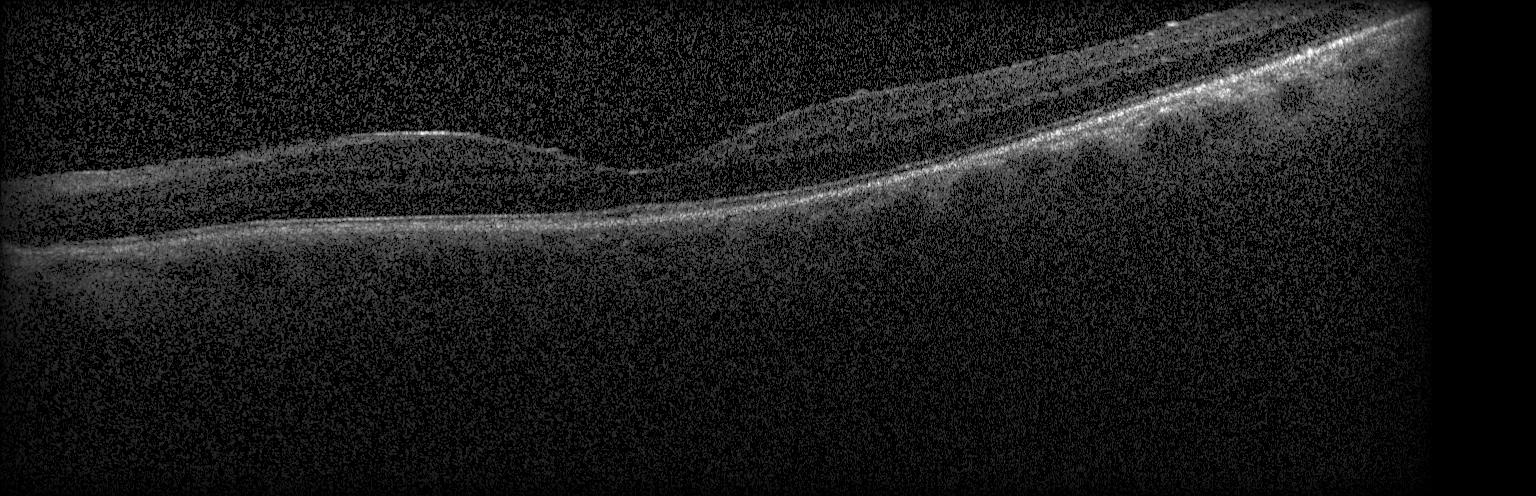

Spectral-domain OCT, macular scan, acquired on a Heidelberg Spectralis, optical coherence tomography B-scan. Macular OCT: no choroidal neovascularization, diabetic macular edema, or drusen.